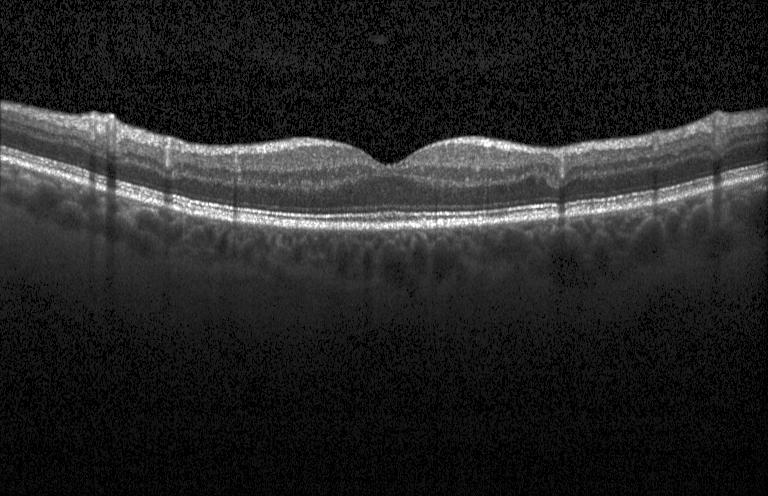 Macular OCT demonstrating no evidence of CNV, DME, or drusen.